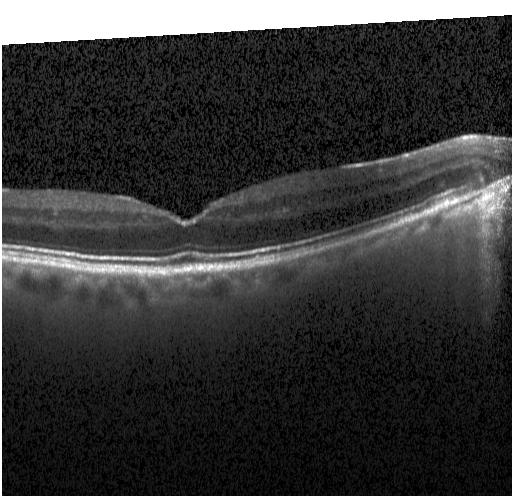

Optical coherence tomography B-scan
Diagnosis: no evidence of CNV, DME, or drusen.